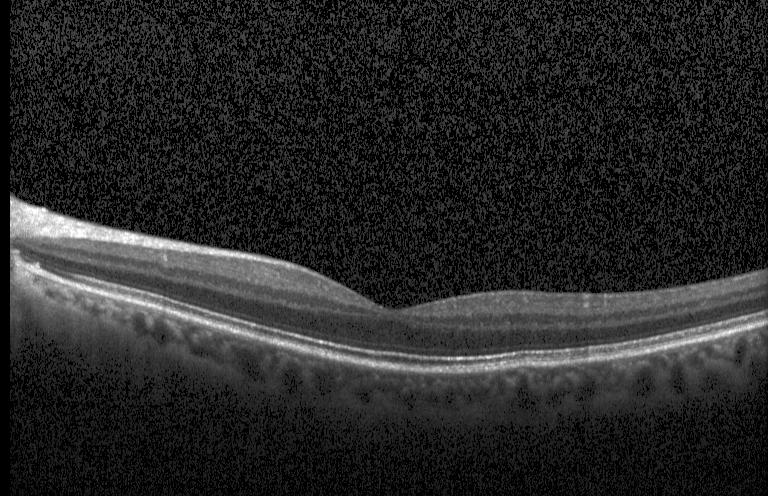
Impression: no choroidal neovascularization, diabetic macular edema, or drusen.